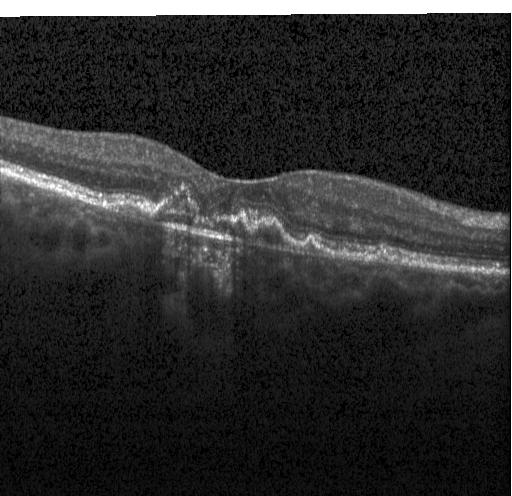 Retinal OCT cross-section, Heidelberg Spectralis
Impression: a choroidal neovascular membrane.